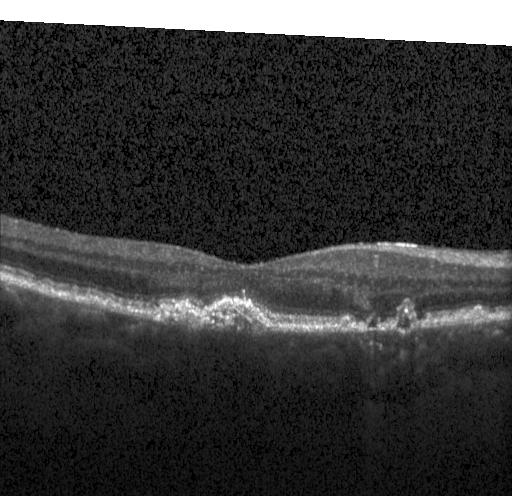

Spectral-domain OCT B-scan: choroidal neovascularization (CNV).